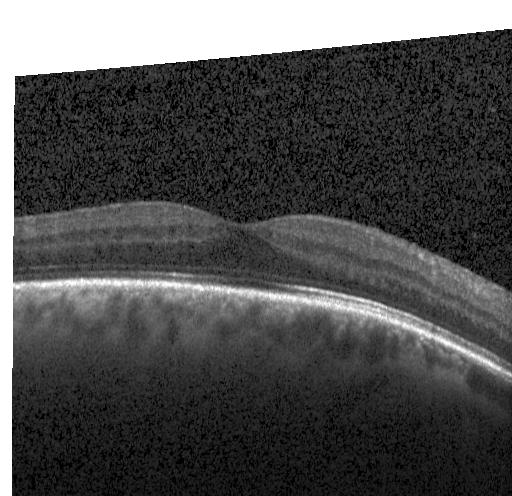
The scan shows no evidence of CNV, DME, or drusen.